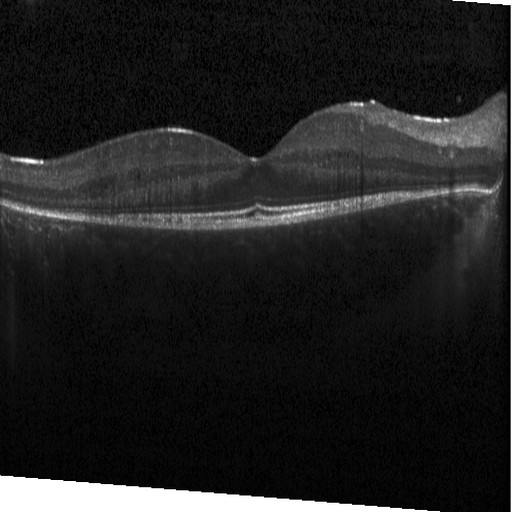

Through the macula, optical coherence tomography B-scan, acquired on a Heidelberg Spectralis.
Macular OCT: diabetic macular edema.